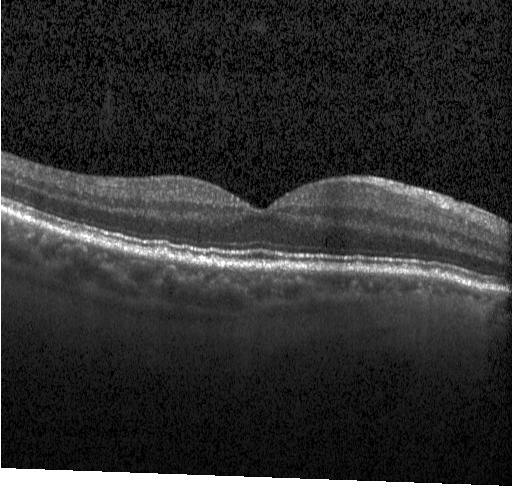 Assessment: drusen.